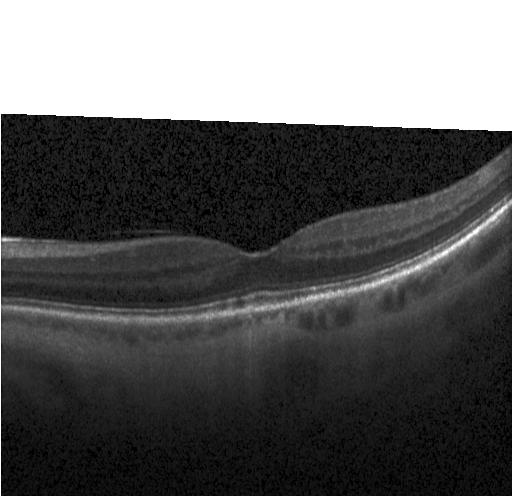
SD-OCT · through the macula · Heidelberg Spectralis OCT system · OCT line scan. No evidence of CNV, DME, or drusen.